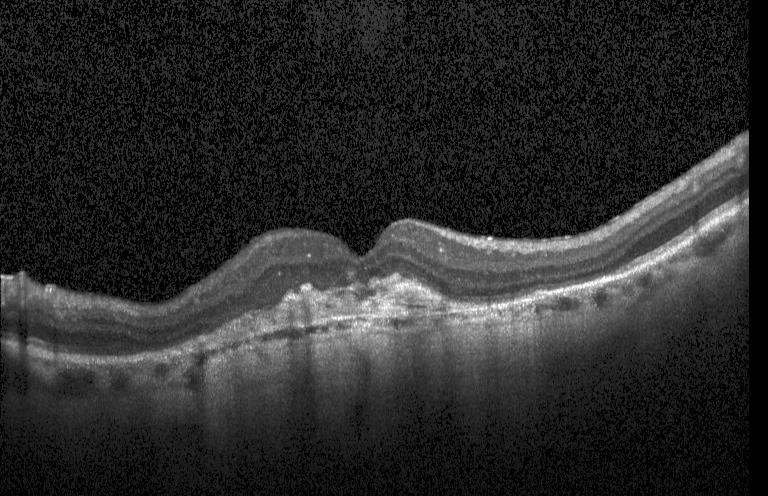 Retinal OCT B-scan, macular scan, spectral-domain optical coherence tomography, Heidelberg Spectralis. CNV.